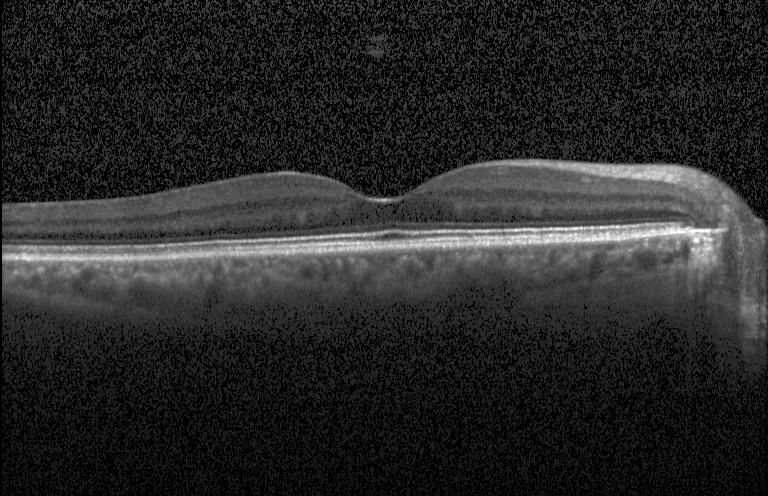 Finding: no choroidal neovascularization, no diabetic macular edema, and no drusen.